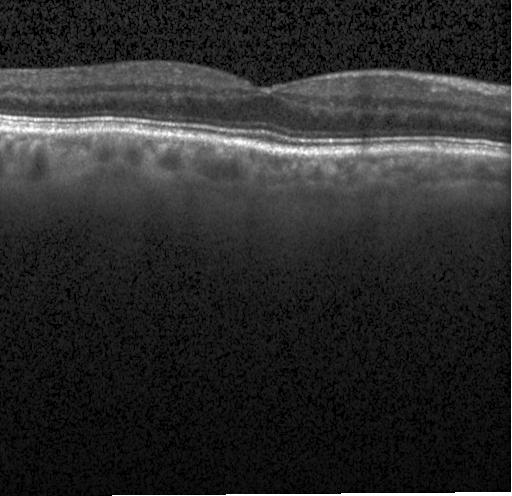 Diagnosis: no evidence of CNV, DME, or drusen.